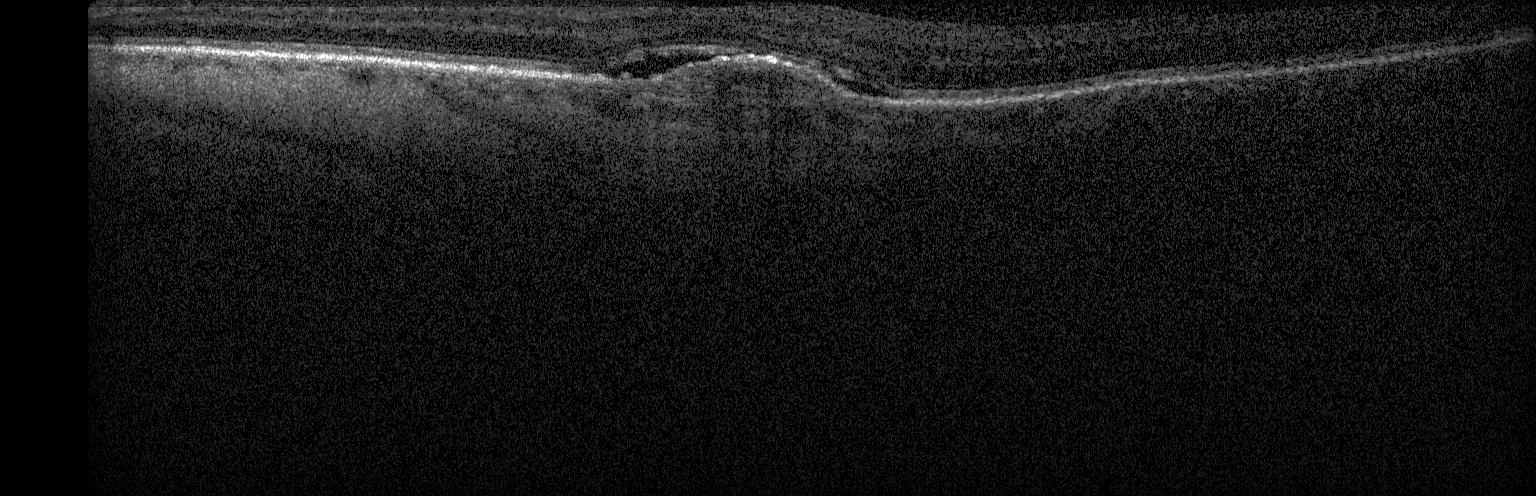
Horizontal scan through the fovea, retinal OCT B-scan — OCT finding: a choroidal neovascular membrane.